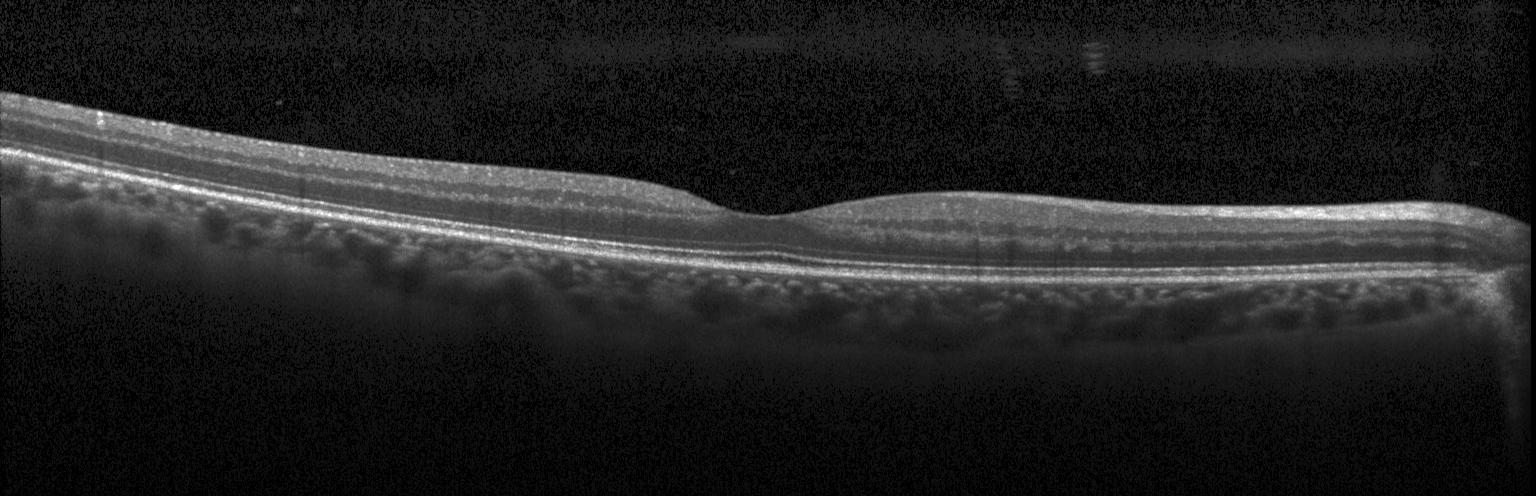
OCT line scan. OCT finding: no evidence of choroidal neovascularization, diabetic macular edema, or drusen.